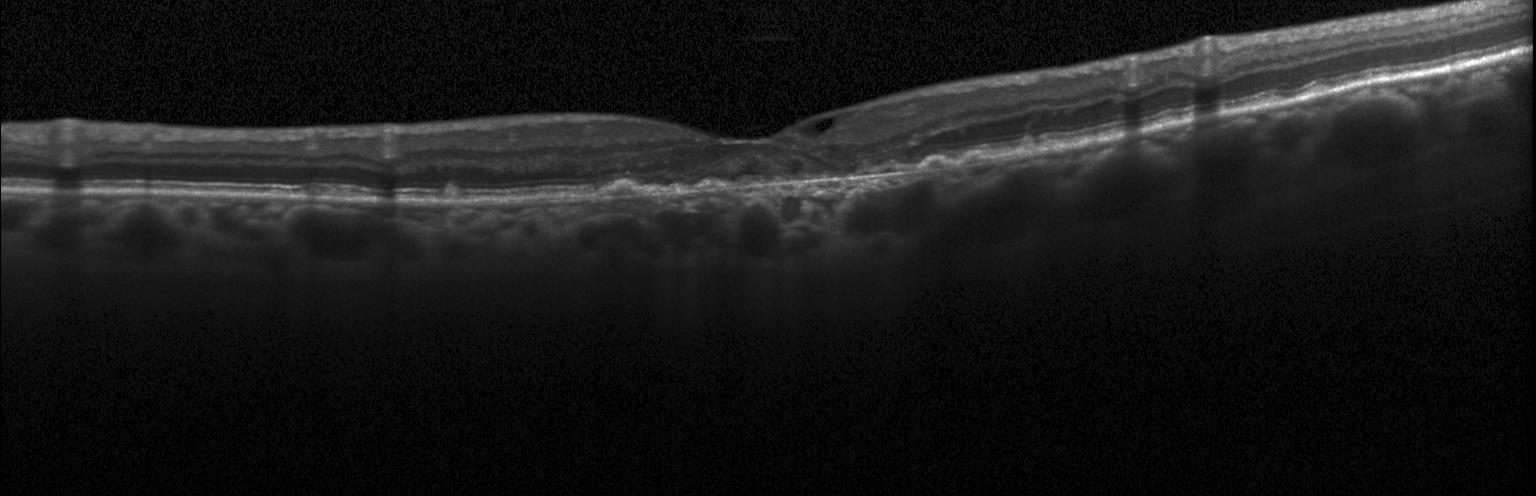

Diagnosis: a choroidal neovascular membrane.